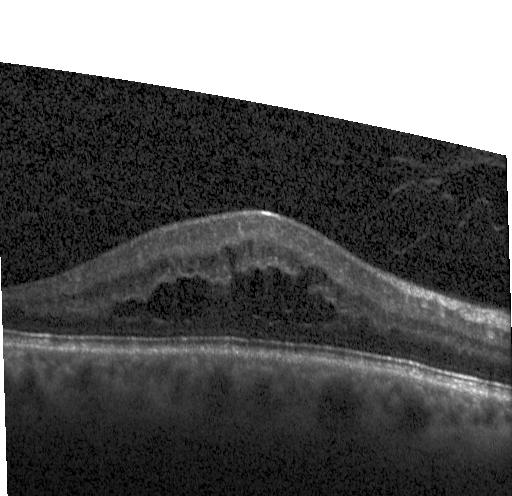
OCT finding: diabetic macular edema (DME).